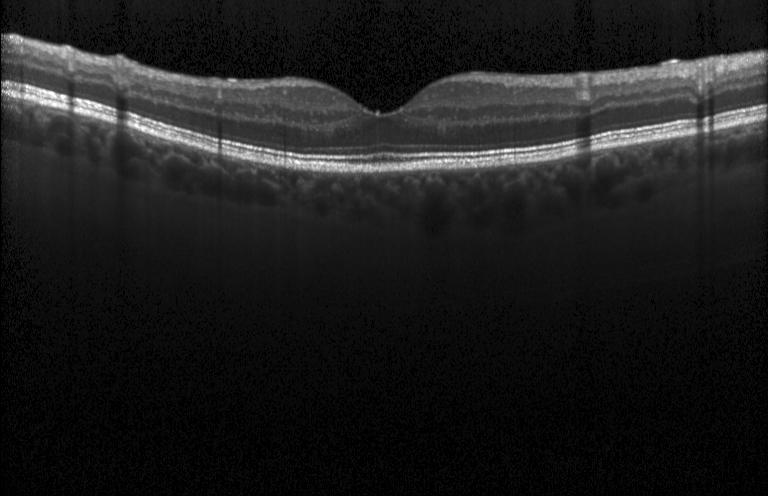

Impression: neither choroidal neovascularization, diabetic macular edema, nor drusen.